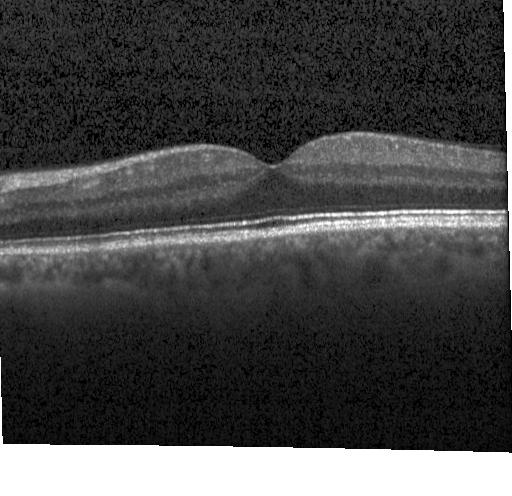
OCT finding: neither choroidal neovascularization, diabetic macular edema, nor drusen.